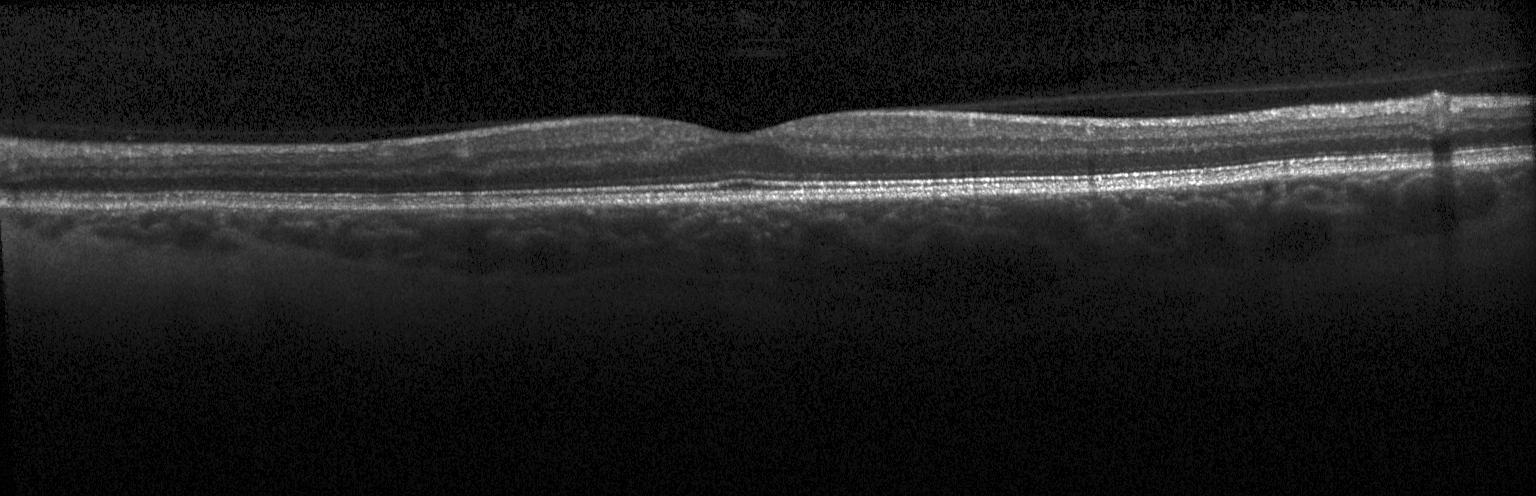
This B-scan demonstrates no evidence of CNV, DME, or drusen.